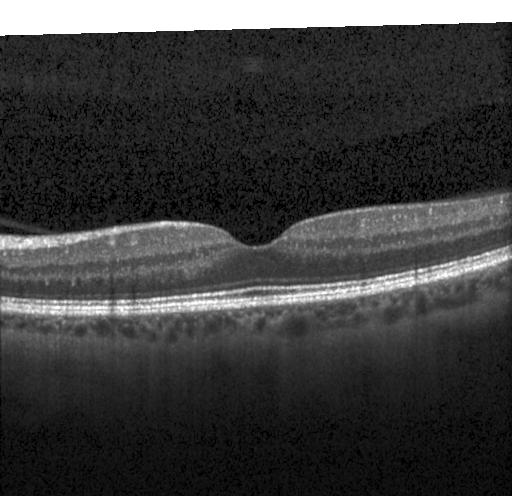 Diagnosis: no choroidal neovascularization, diabetic macular edema, or drusen.